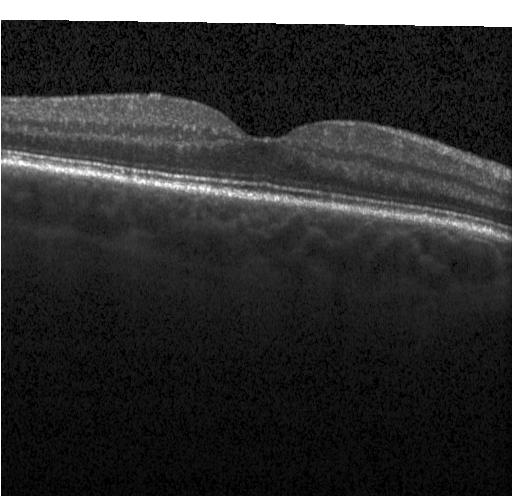
Finding: neither choroidal neovascularization, diabetic macular edema, nor drusen.